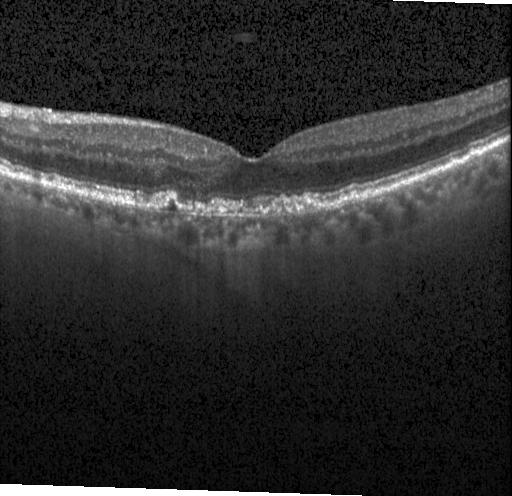
Spectral-domain optical coherence tomography, OCT B-scan. Diagnosis: choroidal neovascularization (CNV).